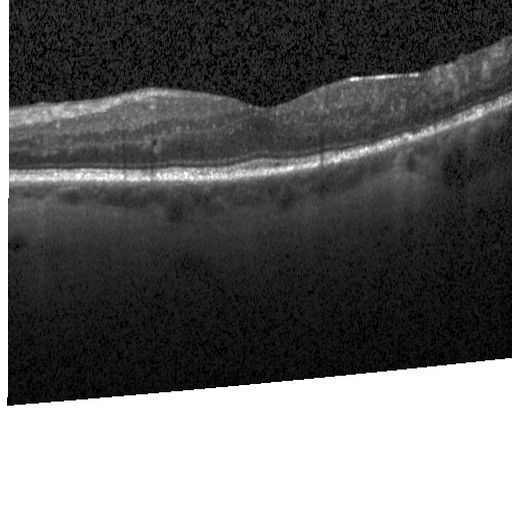
Retinal OCT cross-section — Diagnosis: DME.